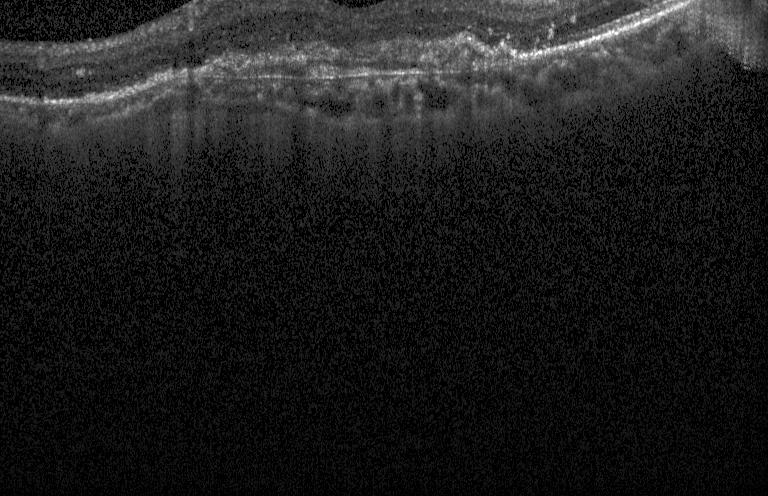 Finding: a choroidal neovascular membrane.